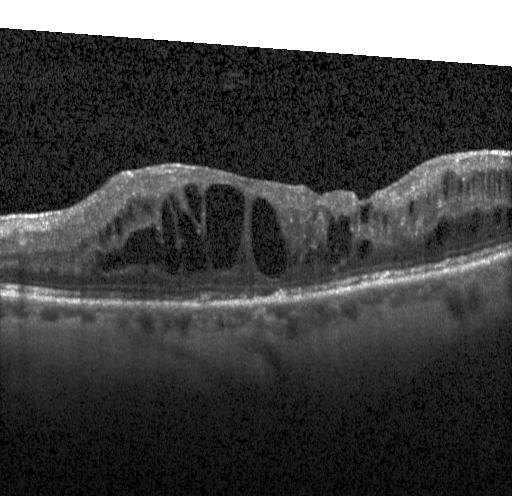 OCT line scan, spectral-domain optical coherence tomography, centered on the fovea.
Impression: diabetic macular edema (DME).